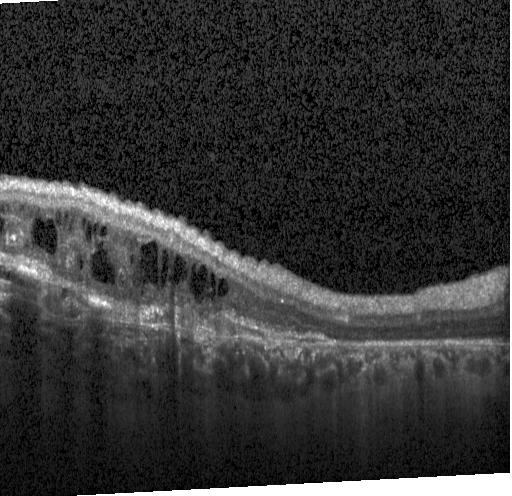
Optical coherence tomography B-scan · fovea-centered · spectral-domain OCT · acquired on a Heidelberg Spectralis. Macular OCT: choroidal neovascularization.